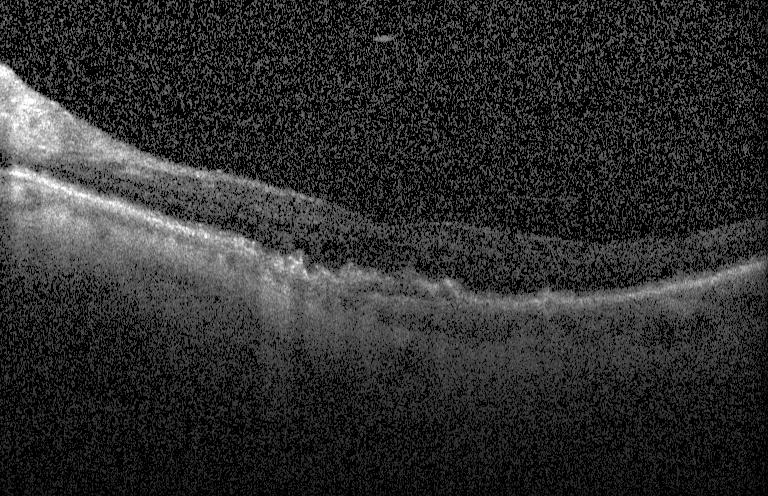 This B-scan demonstrates choroidal neovascularization (CNV).